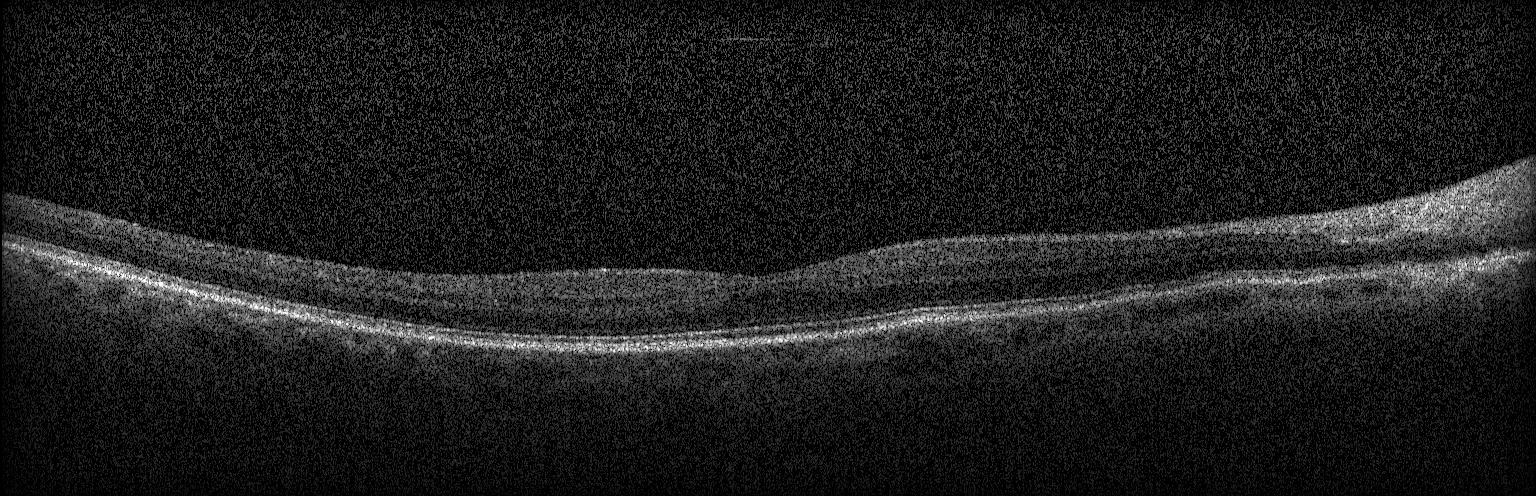 No choroidal neovascularization, no diabetic macular edema, and no drusen.